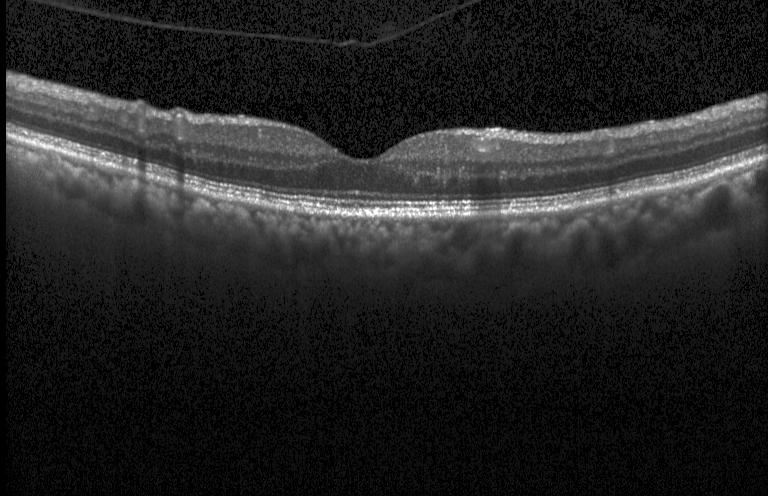 Retinal OCT cross-section; fovea-centered; spectral-domain optical coherence tomography.
Diagnosis: no choroidal neovascularization, no diabetic macular edema, and no drusen.